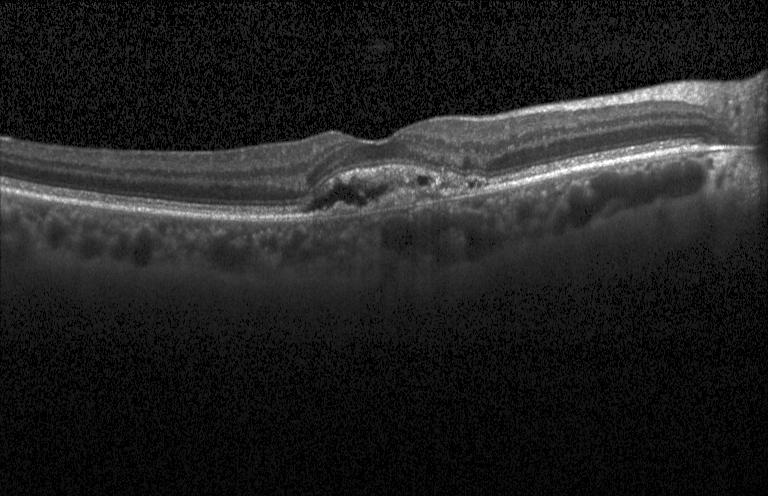
Spectral-domain optical coherence tomography; optical coherence tomography B-scan
Diagnosis: CNV.